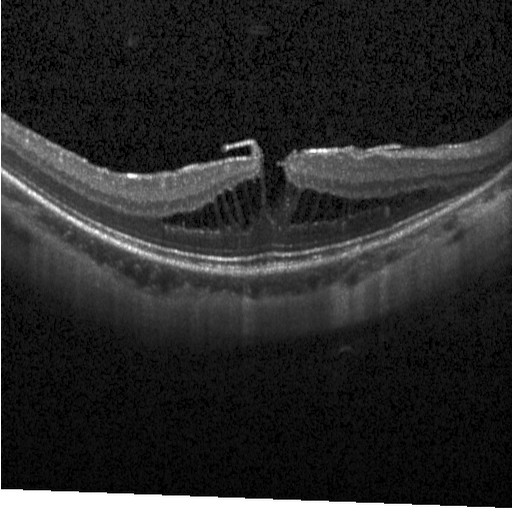

Heidelberg Spectralis OCT system. Spectral-domain OCT. Optical coherence tomography scan. Through the macula — This B-scan demonstrates DME.